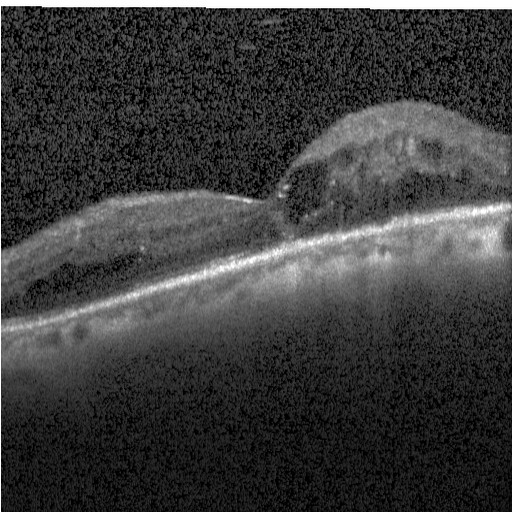 Diagnosis: diabetic macular edema.